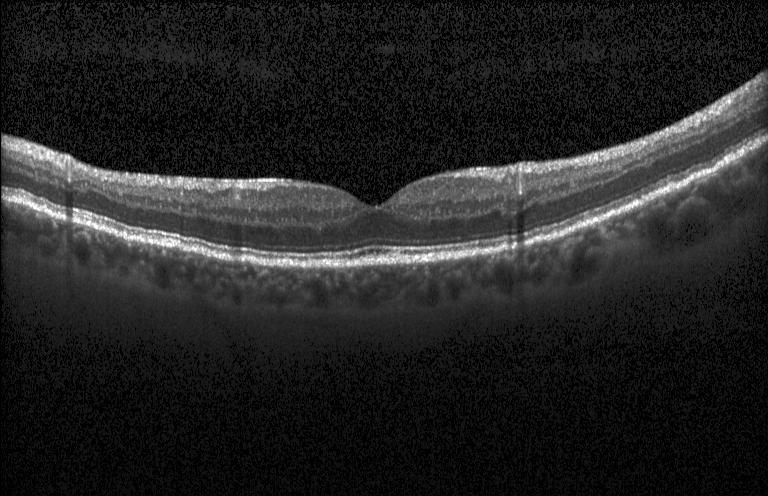 Finding: neither CNV, DME, nor drusen.